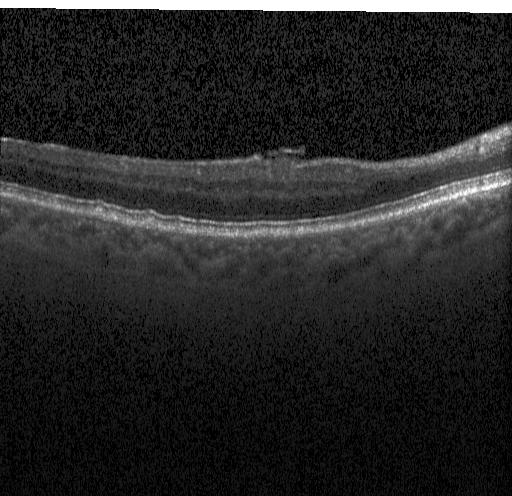

Dx: sub-RPE drusenoid deposits.